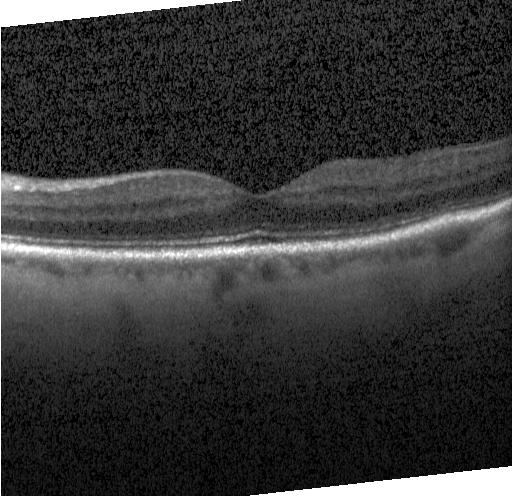
Instrument: Heidelberg Spectralis. Optical coherence tomography scan — Impression: no CNV, no DME, and no drusen.